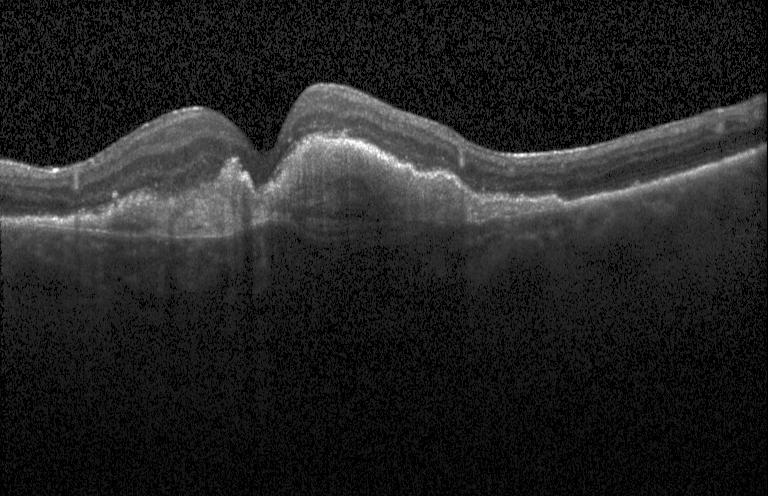
OCT B-scan.
OCT finding: a choroidal neovascular membrane.